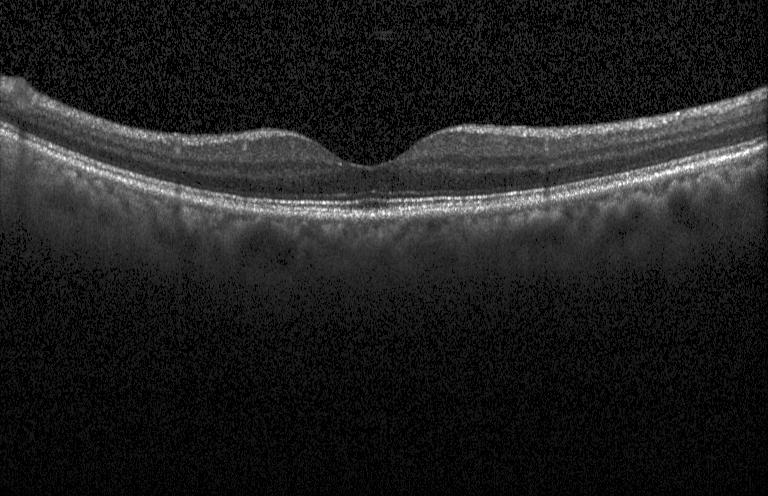

Retinal OCT cross-section; horizontal scan through the fovea; spectral-domain optical coherence tomography. This B-scan demonstrates no choroidal neovascularization, no diabetic macular edema, and no drusen.